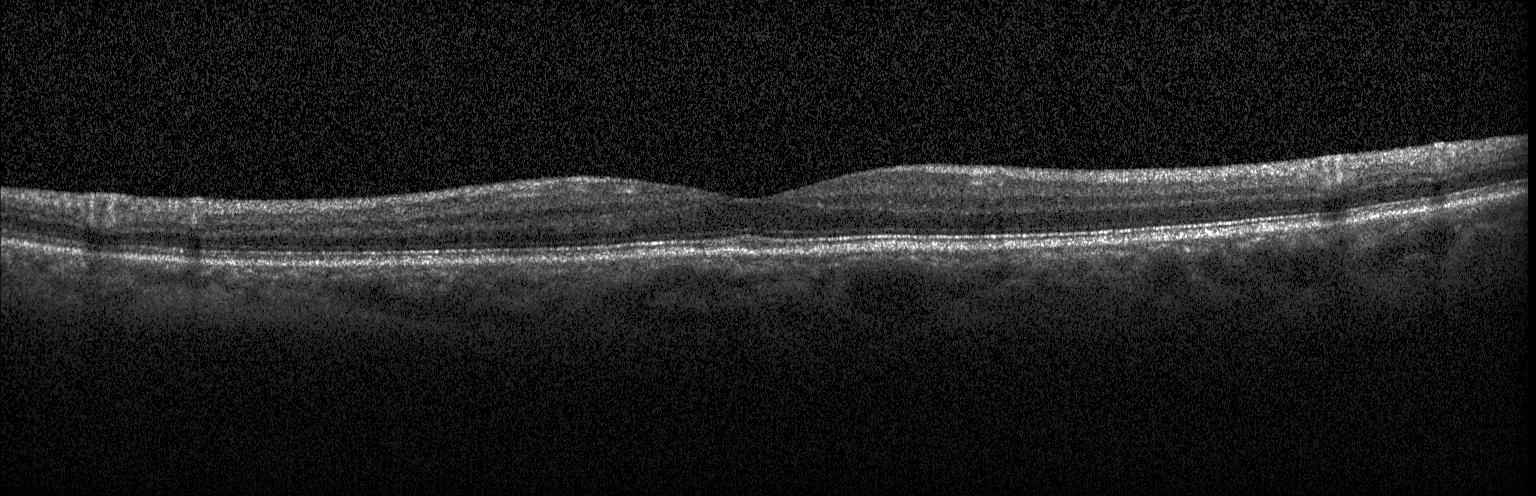 SD-OCT. Instrument: Heidelberg Spectralis. OCT line scan.
Neither CNV, DME, nor drusen.